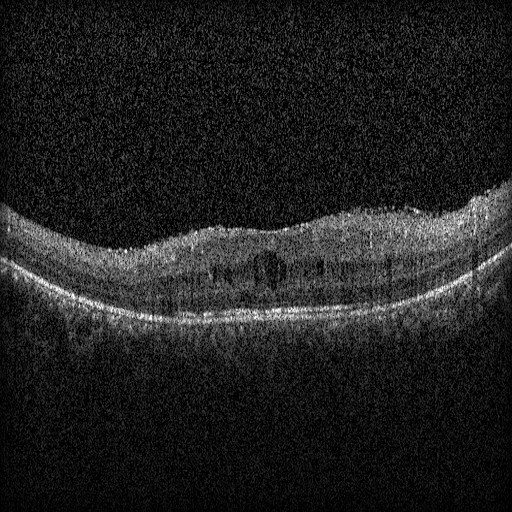

Spectral-domain optical coherence tomography; optical coherence tomography scan; macular scan; acquired on a Heidelberg Spectralis
This B-scan demonstrates diabetic macular edema (DME).